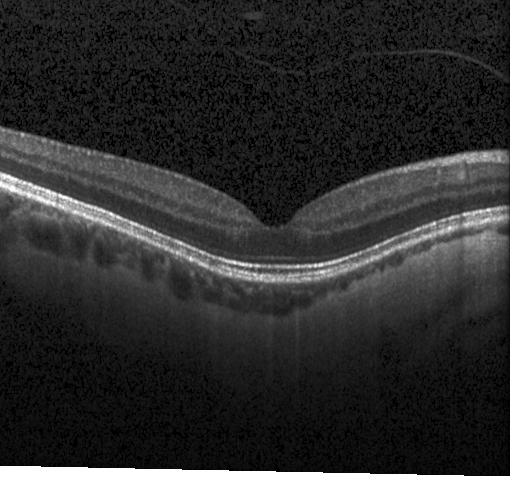
Horizontal scan through the fovea, spectral-domain optical coherence tomography, OCT line scan, acquired on a Heidelberg Spectralis. No evidence of CNV, DME, or drusen.